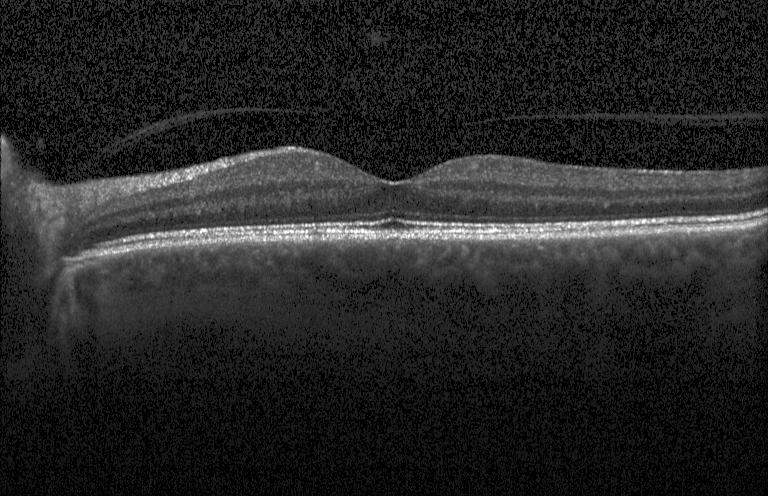

Spectral-domain optical coherence tomography; OCT B-scan — Impression: neither choroidal neovascularization, diabetic macular edema, nor drusen.